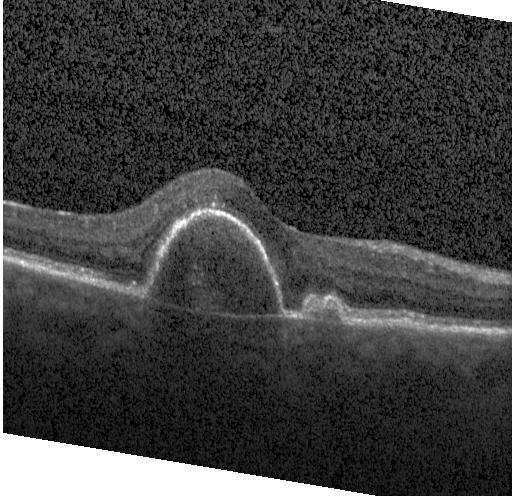 Optical coherence tomography scan · instrument: Heidelberg Spectralis · spectral-domain OCT
A choroidal neovascular membrane.